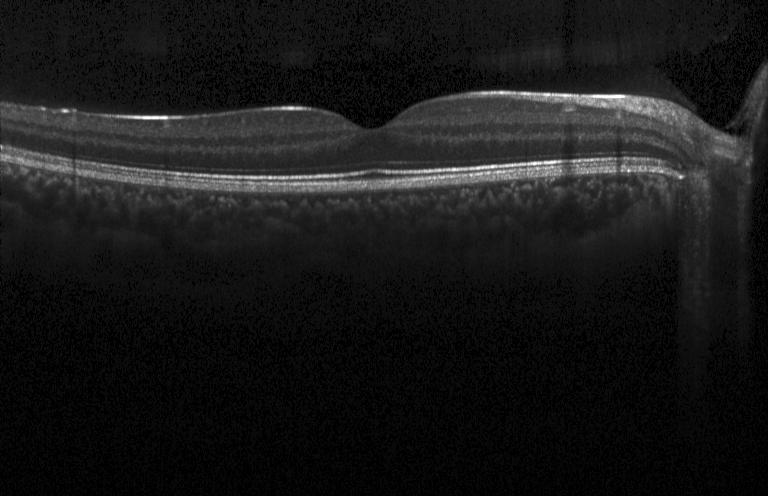

Diagnosis: no choroidal neovascularization, diabetic macular edema, or drusen.